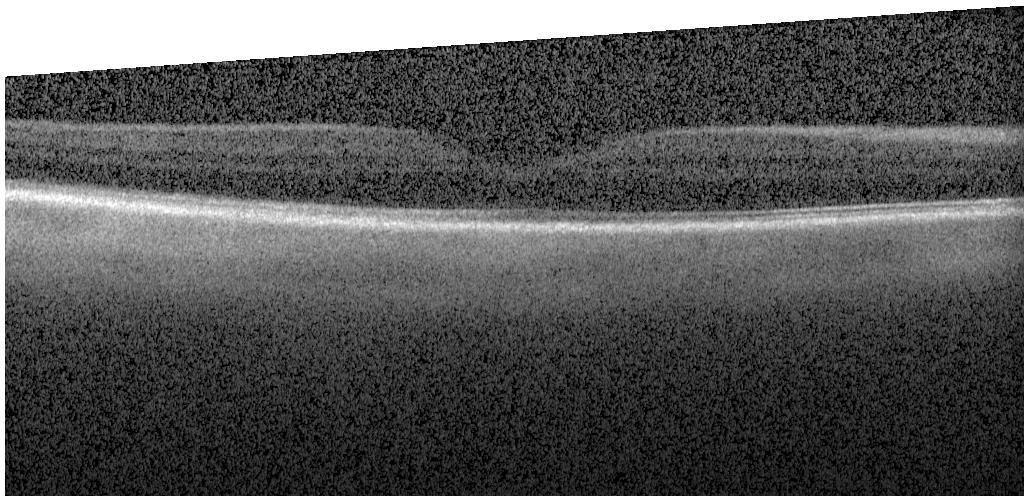 OCT line scan, acquired on a Heidelberg Spectralis, spectral-domain OCT.
This B-scan demonstrates no evidence of choroidal neovascularization, diabetic macular edema, or drusen.